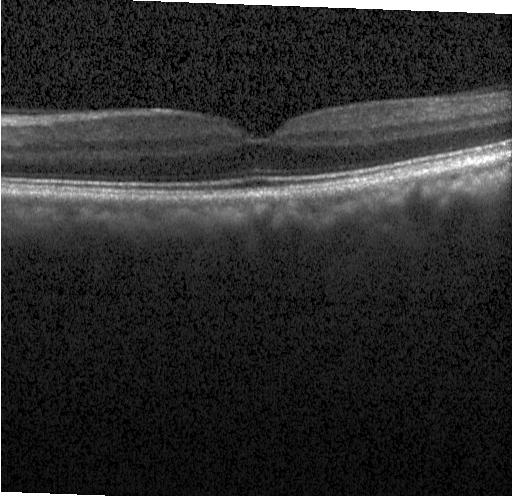
OCT B-scan
Assessment: no evidence of choroidal neovascularization, diabetic macular edema, or drusen.